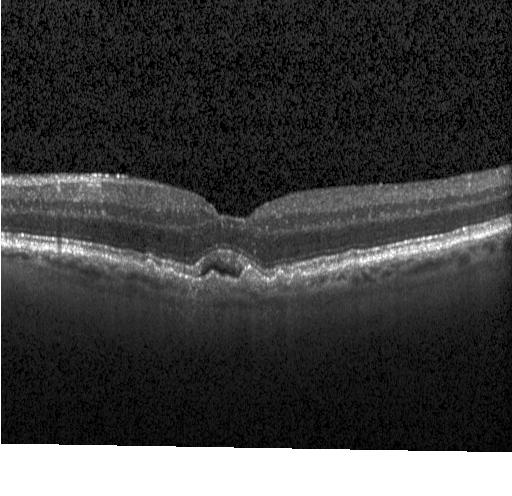 OCT B-scan · horizontal scan through the fovea · spectral-domain OCT
Finding: choroidal neovascularization (CNV).